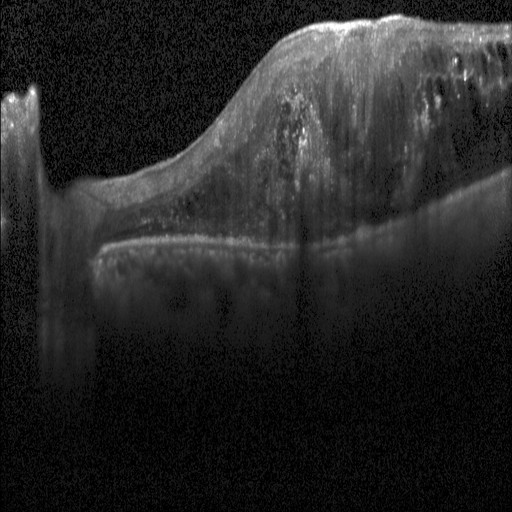

Retinal OCT cross-section. Through the macula
OCT finding: diabetic macular edema (DME).